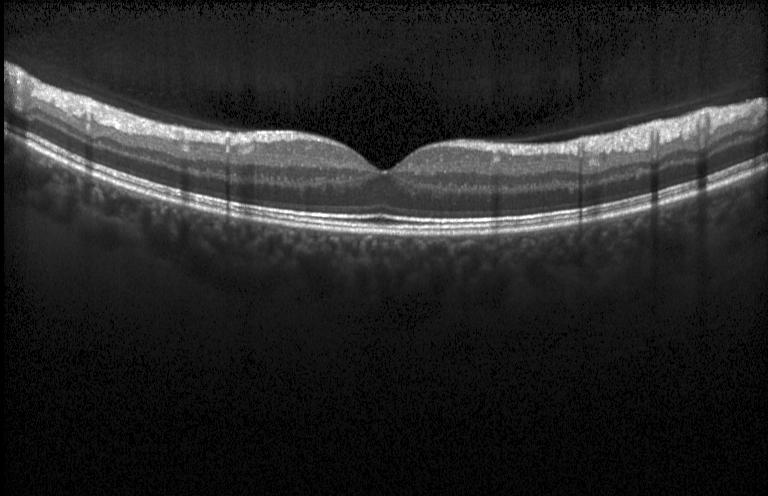 No choroidal neovascularization, diabetic macular edema, or drusen.